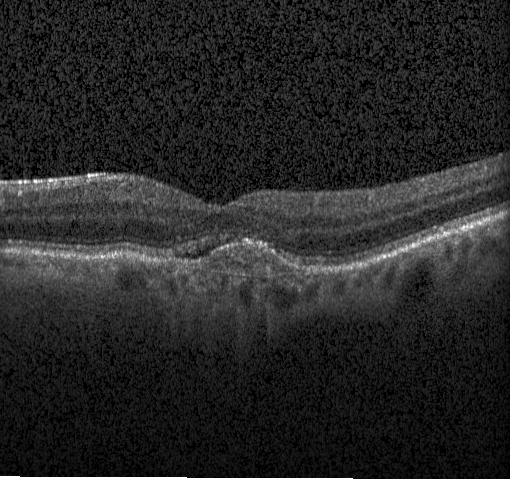

OCT B-scan. Finding: CNV.